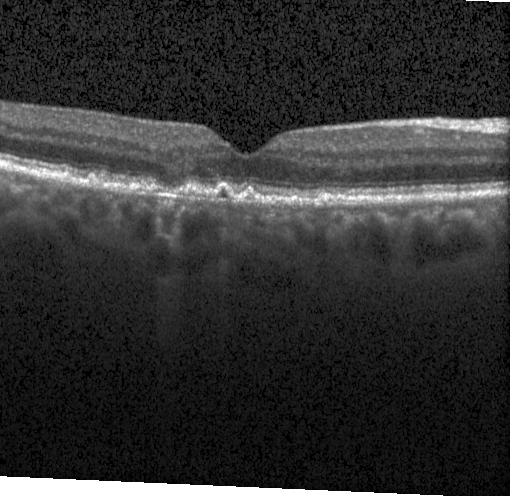

Spectral-domain OCT. OCT line scan. Macular scan. Instrument: Heidelberg Spectralis
Diagnosis: a choroidal neovascular membrane.